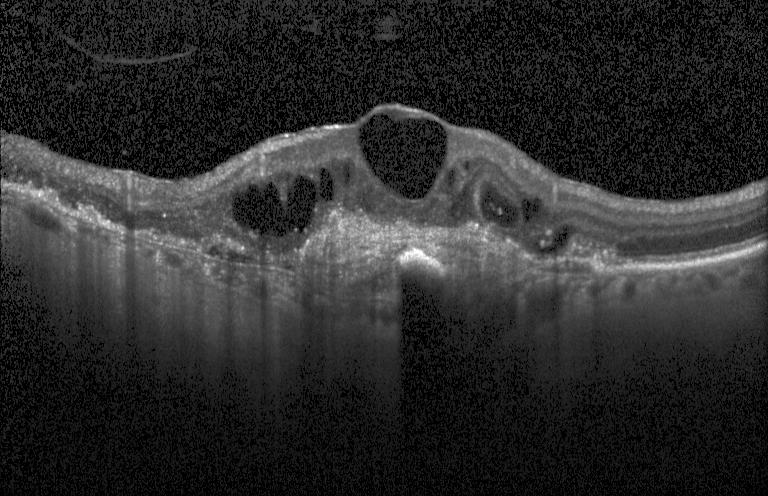
This B-scan demonstrates choroidal neovascularization.